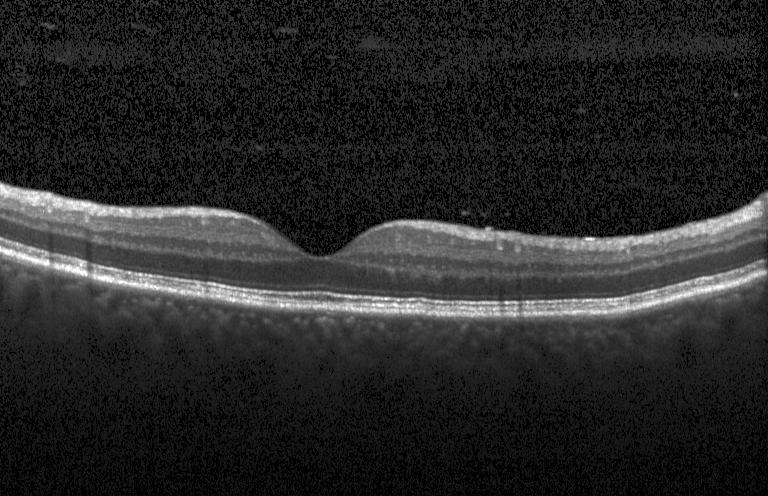

The scan shows no evidence of choroidal neovascularization, diabetic macular edema, or drusen.